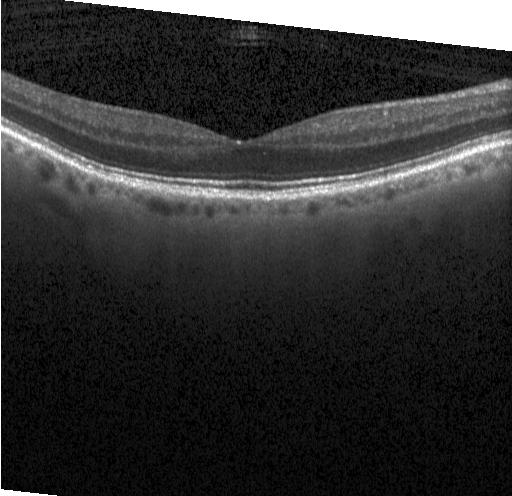 Retinal OCT B-scan. The scan shows no choroidal neovascularization, diabetic macular edema, or drusen.